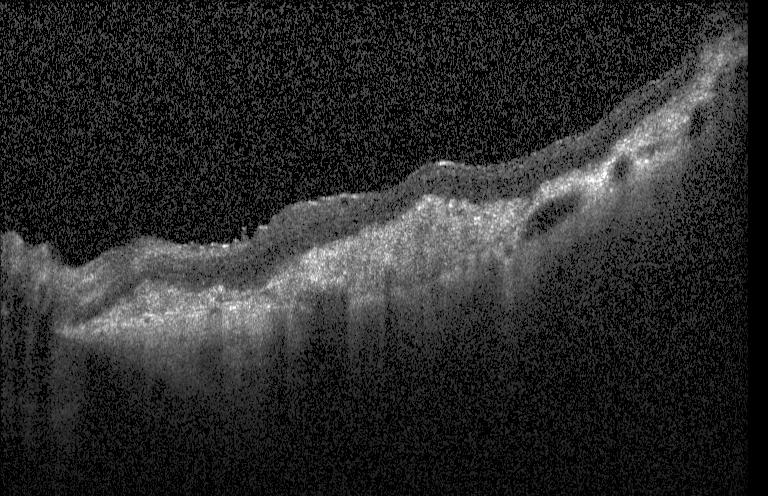 Spectral-domain OCT · optical coherence tomography B-scan — Impression: choroidal neovascularization.